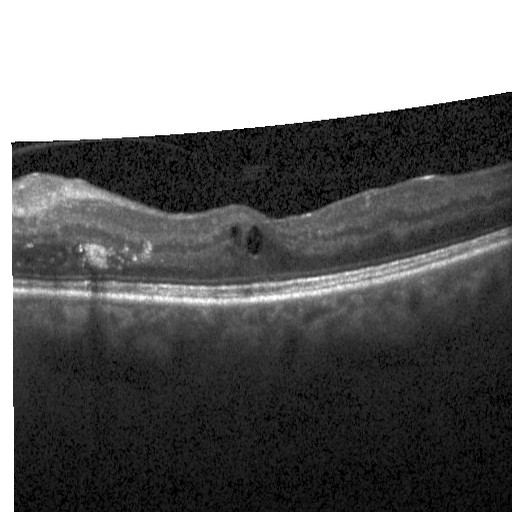 OCT line scan.
Finding: DME.